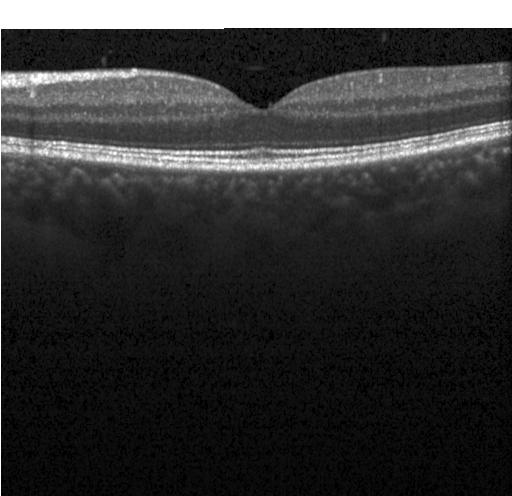

Heidelberg Spectralis · SD-OCT · centered on the fovea · optical coherence tomography scan — No choroidal neovascularization, diabetic macular edema, or drusen.